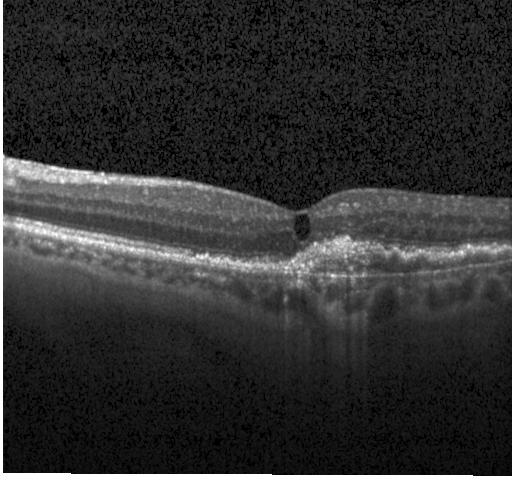 Impression: a choroidal neovascular membrane.